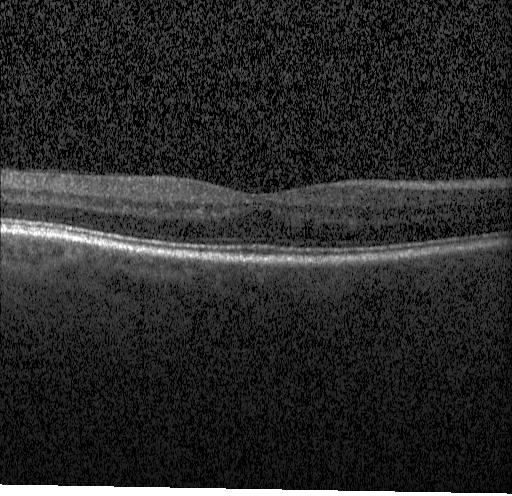 Spectral-domain OCT B-scan: no choroidal neovascularization, no diabetic macular edema, and no drusen.